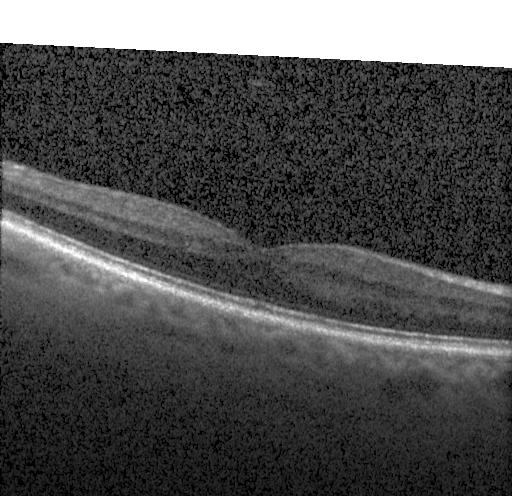 Finding: no evidence of choroidal neovascularization, diabetic macular edema, or drusen.